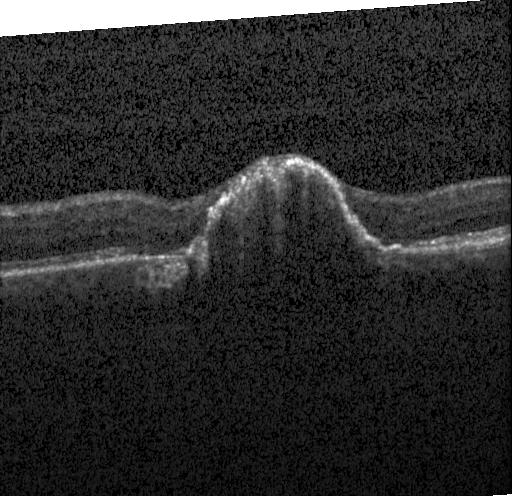
Fovea-centered · retinal OCT B-scan · Heidelberg Spectralis OCT system.
OCT finding: choroidal neovascularization (CNV).